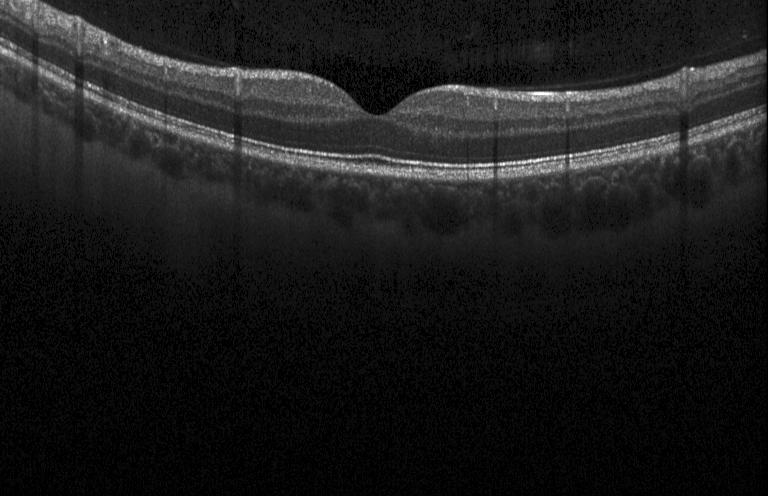 Heidelberg Spectralis OCT system · retinal OCT cross-section · SD-OCT
Diagnosis: no evidence of choroidal neovascularization, diabetic macular edema, or drusen.